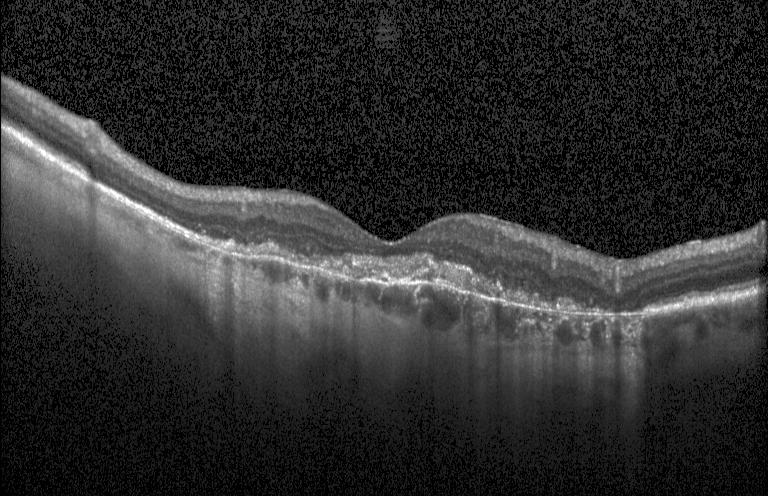

Retinal OCT cross-section. Spectral-domain optical coherence tomography. OCT finding: a choroidal neovascular membrane.